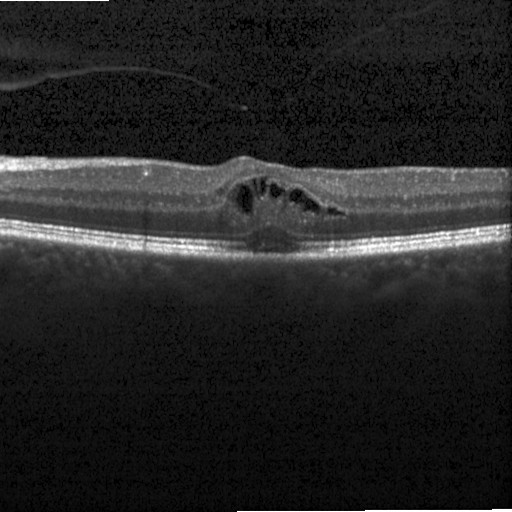

Macular OCT demonstrating diabetic macular edema (DME).